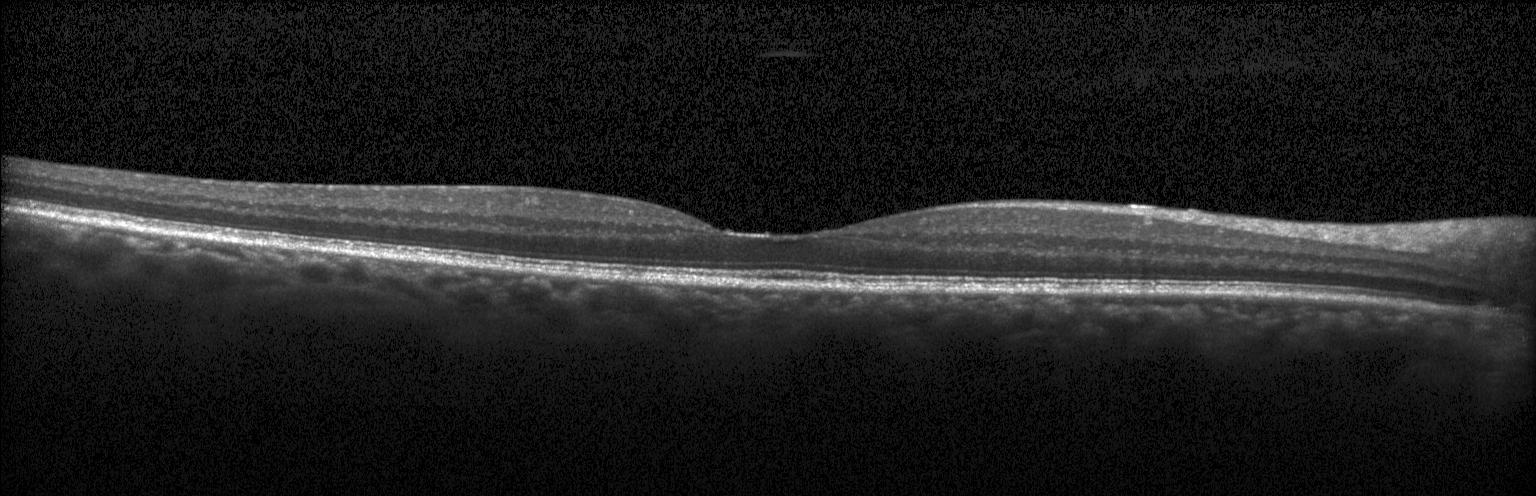

Optical coherence tomography scan · Heidelberg Spectralis · SD-OCT — This B-scan demonstrates neither choroidal neovascularization, diabetic macular edema, nor drusen.